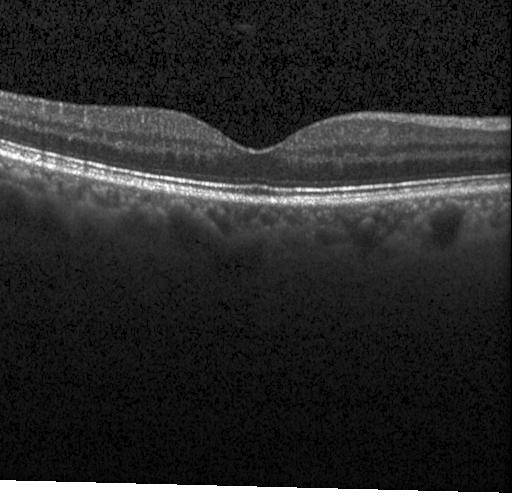

Dx: no evidence of choroidal neovascularization, diabetic macular edema, or drusen.